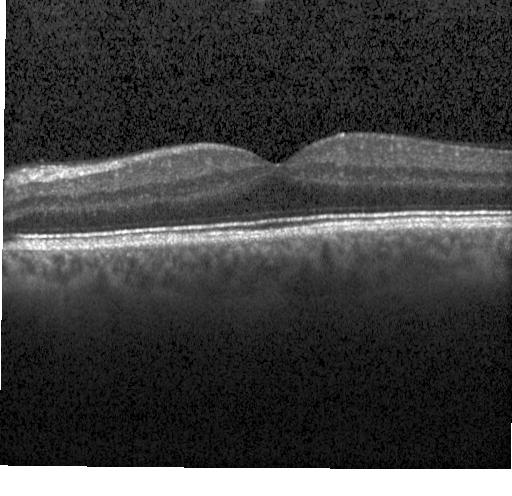
Retinal OCT cross-section. Heidelberg Spectralis OCT system. Spectral-domain optical coherence tomography.
Neither CNV, DME, nor drusen.